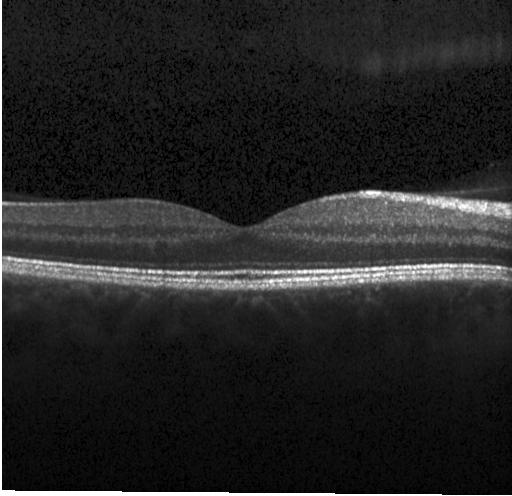
Finding: no evidence of CNV, DME, or drusen.